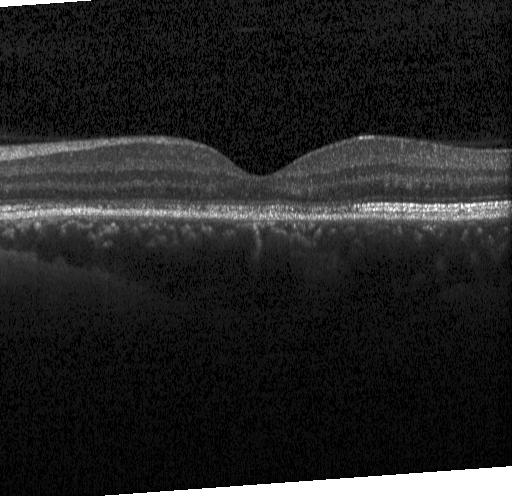

Impression: no evidence of choroidal neovascularization, diabetic macular edema, or drusen.